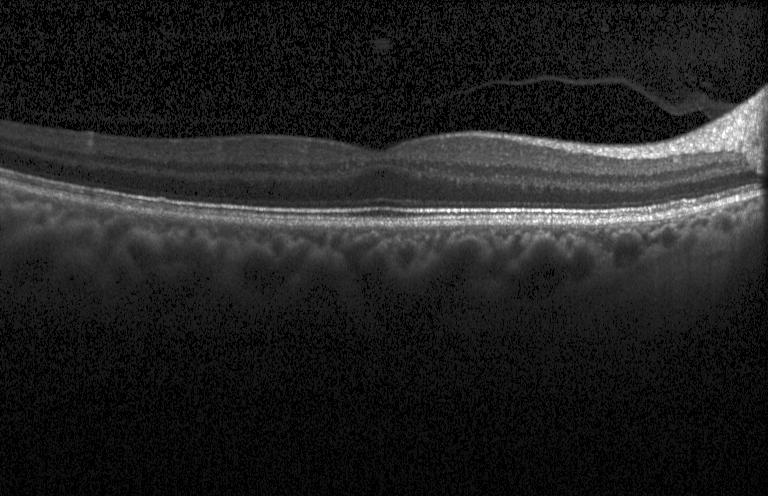
Spectral-domain optical coherence tomography, optical coherence tomography scan, fovea-centered, Heidelberg Spectralis OCT system.
Impression: no choroidal neovascularization, diabetic macular edema, or drusen.